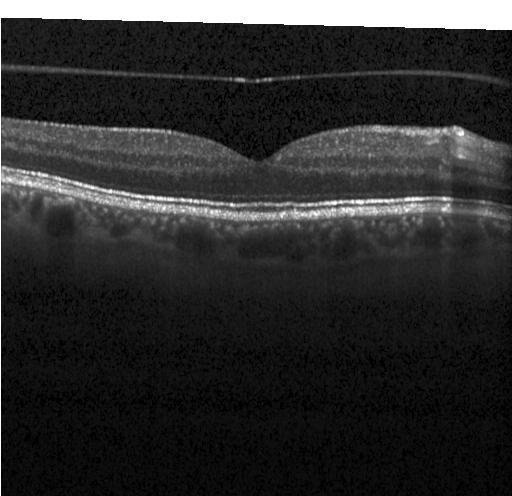

The scan shows no CNV, DME, or drusen.